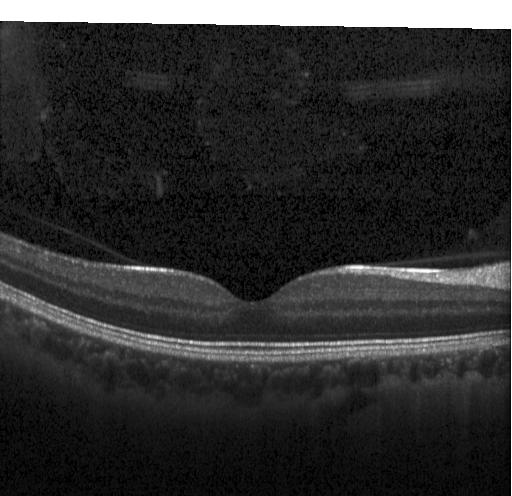
Spectral-domain OCT B-scan: no evidence of CNV, DME, or drusen.